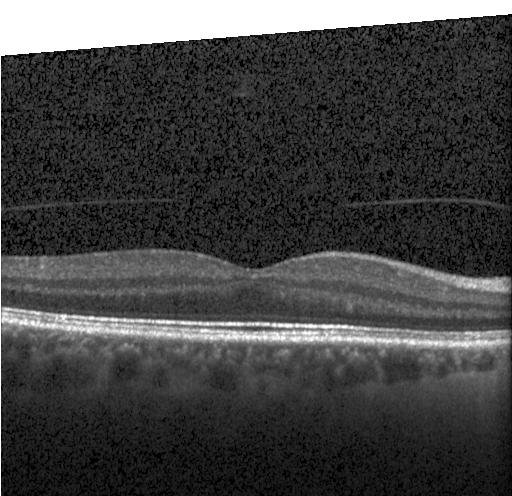

OCT B-scan showing no evidence of CNV, DME, or drusen.